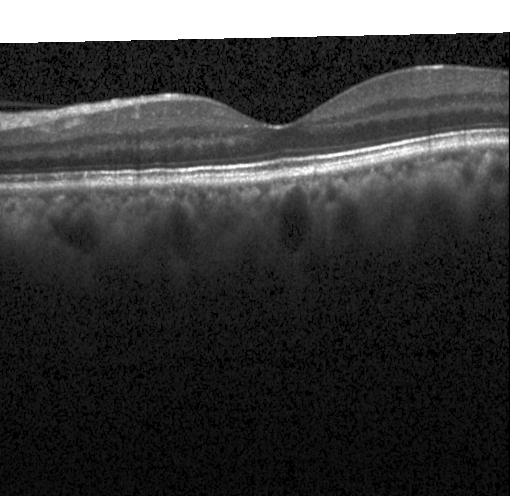
Retinal OCT cross-section. SD-OCT. Through the macula
Finding: no choroidal neovascularization, no diabetic macular edema, and no drusen.